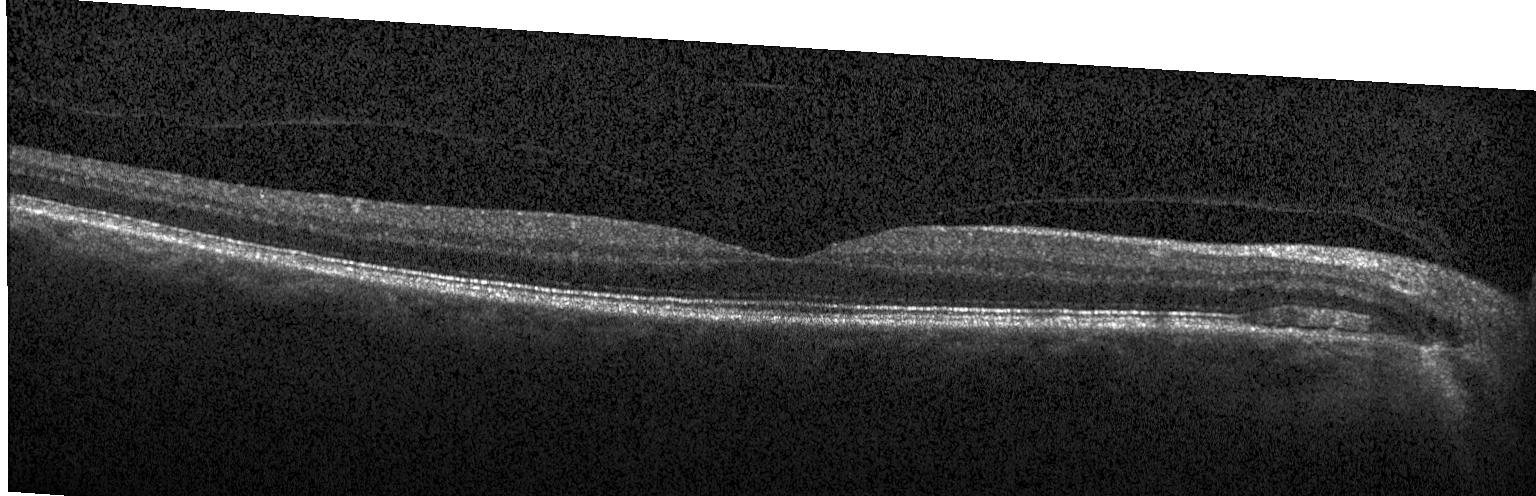 Optical coherence tomography B-scan — Finding: neither choroidal neovascularization, diabetic macular edema, nor drusen.